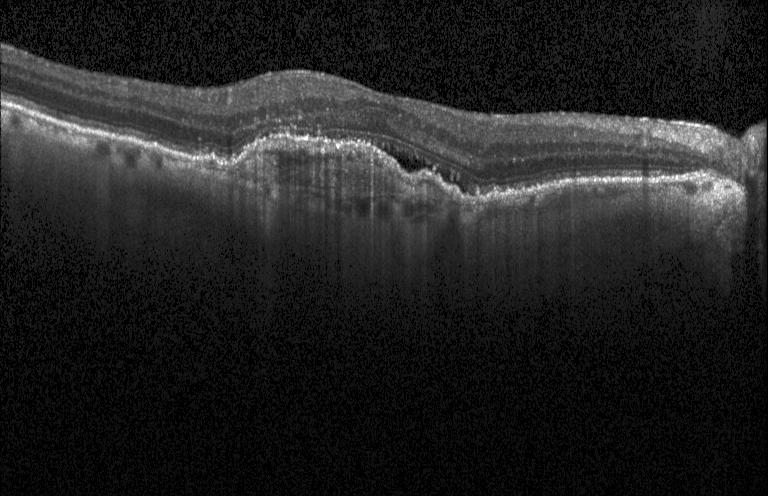

SD-OCT · Heidelberg Spectralis OCT system · macular scan · OCT line scan. Finding: a choroidal neovascular membrane.